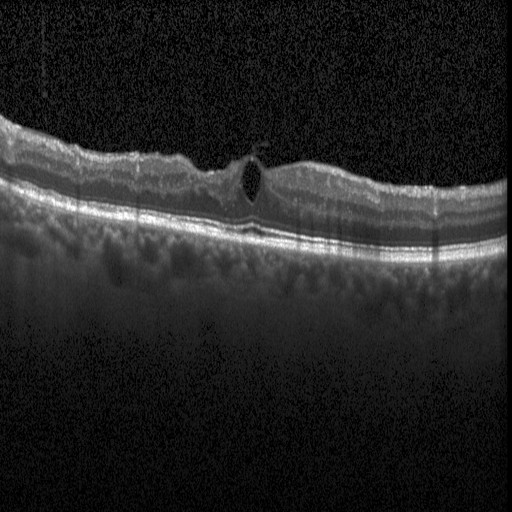

Finding: diabetic macular edema.